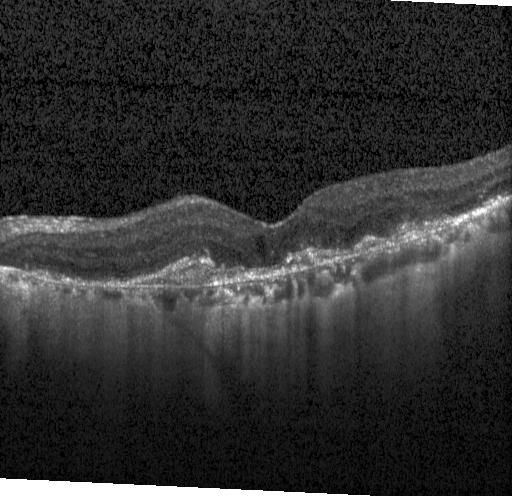 OCT B-scan. OCT finding: CNV.